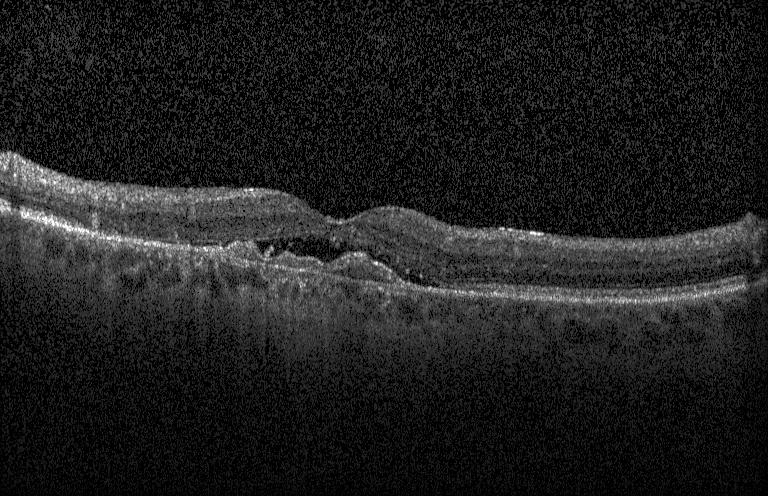

OCT finding: choroidal neovascularization (CNV).